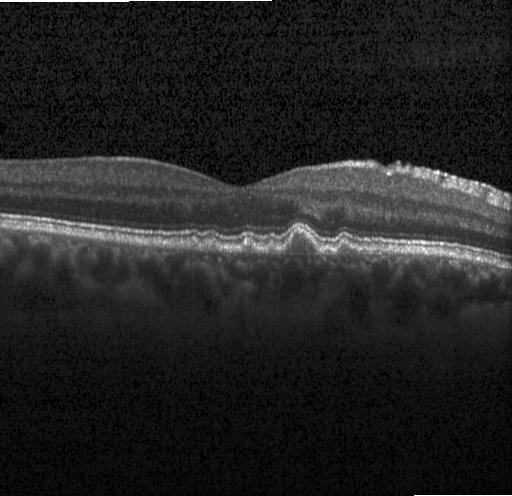
Retinal OCT cross-section. Heidelberg Spectralis
Impression: multiple drusen.